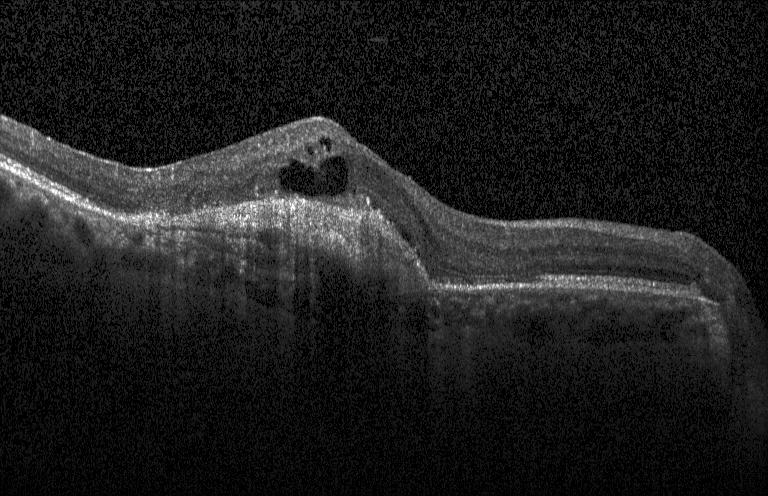 A choroidal neovascular membrane.